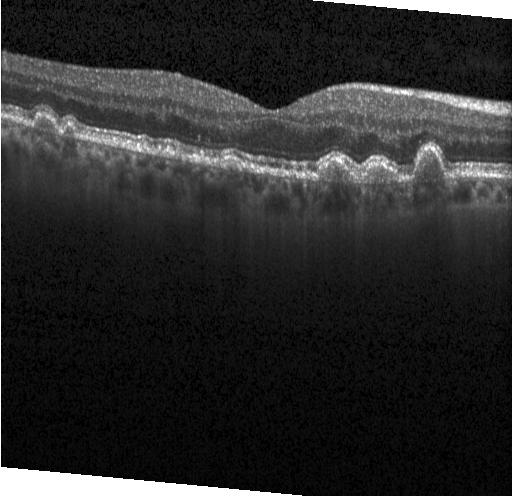
Retinal OCT B-scan · spectral-domain optical coherence tomography.
Dx: sub-RPE drusenoid deposits.